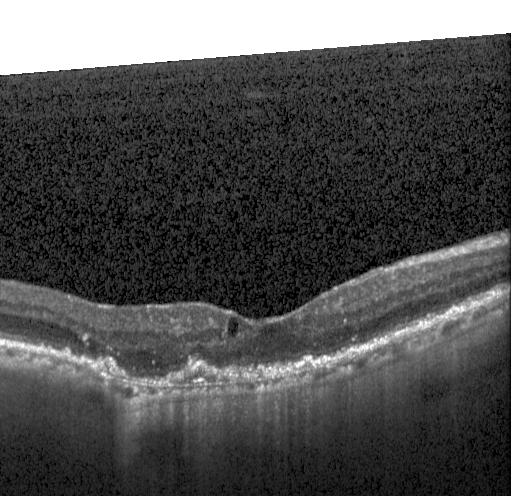
Macular OCT demonstrating a choroidal neovascular membrane.